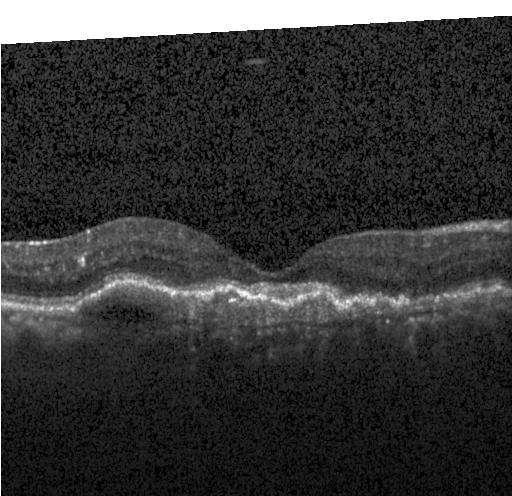 Optical coherence tomography B-scan · instrument: Heidelberg Spectralis · through the macula.
Diagnosis: CNV.